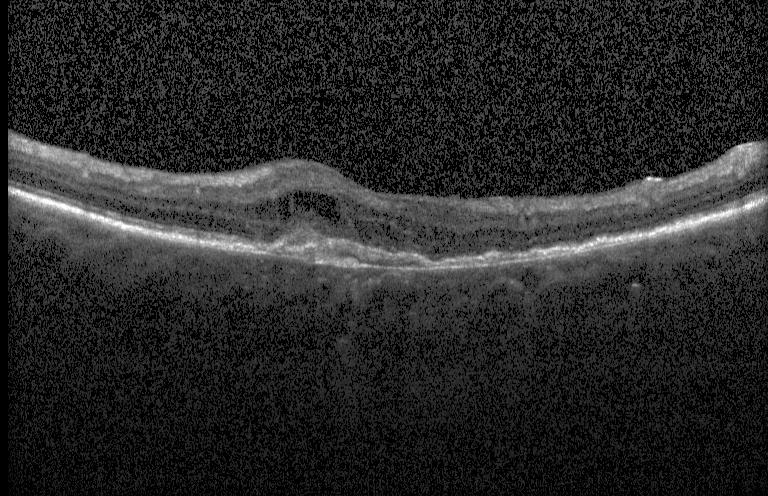
Optical coherence tomography scan. Diagnosis: a choroidal neovascular membrane.